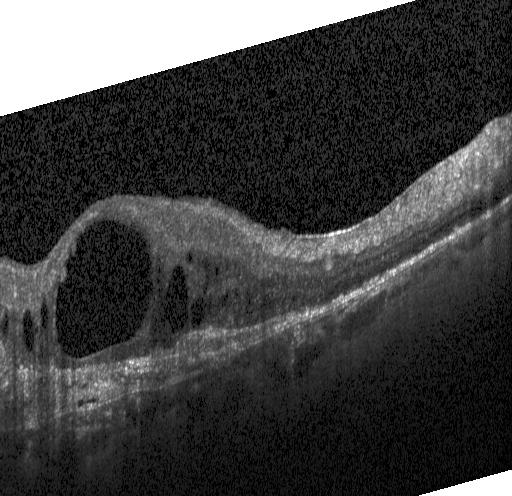 Finding: choroidal neovascularization (CNV).